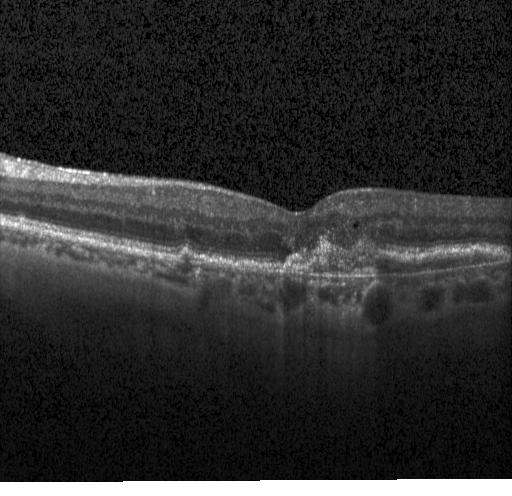

Instrument: Heidelberg Spectralis; SD-OCT; retinal OCT B-scan — Choroidal neovascularization.